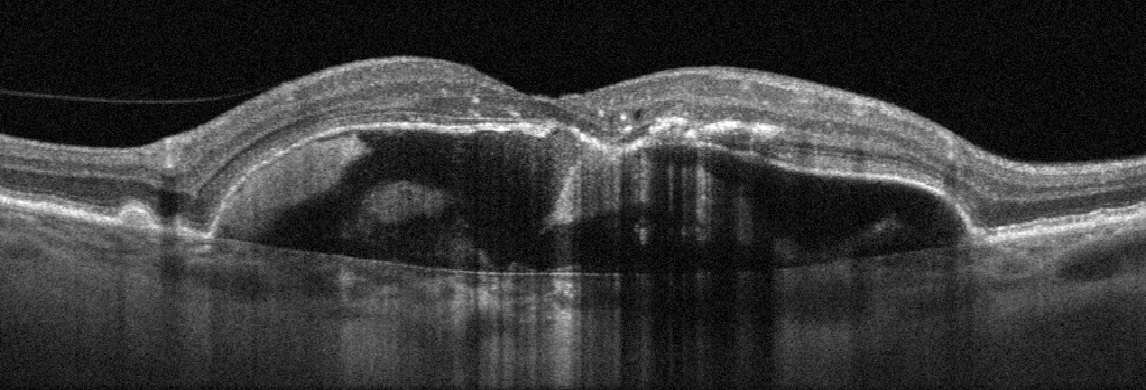
Impression: AMD.